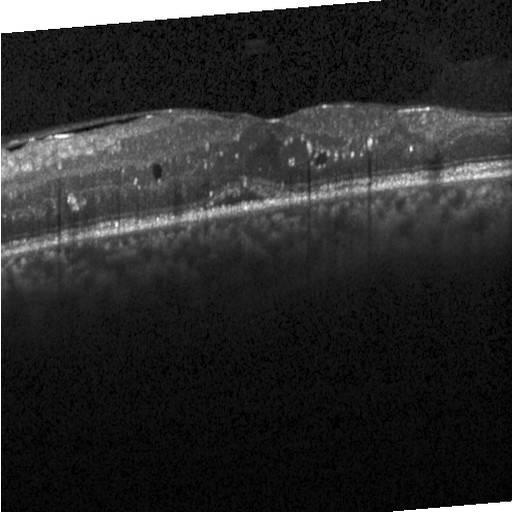
Optical coherence tomography scan. Diagnosis: diabetic macular edema (DME).